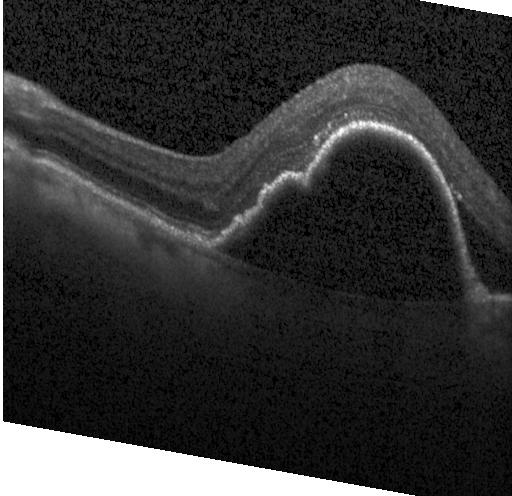

Spectral-domain optical coherence tomography. OCT line scan. Choroidal neovascularization.